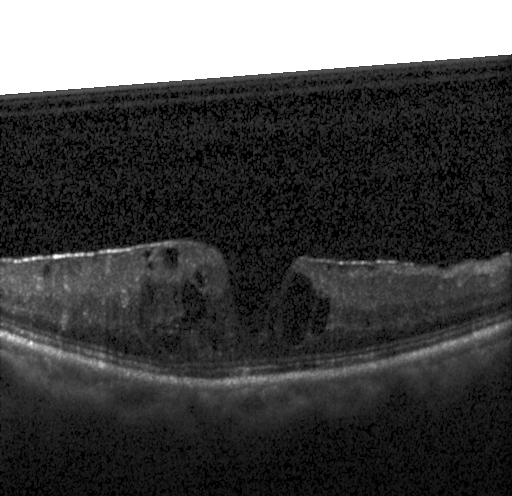 Retinal OCT cross-section · instrument: Heidelberg Spectralis · spectral-domain optical coherence tomography. Assessment: diabetic macular edema (DME).